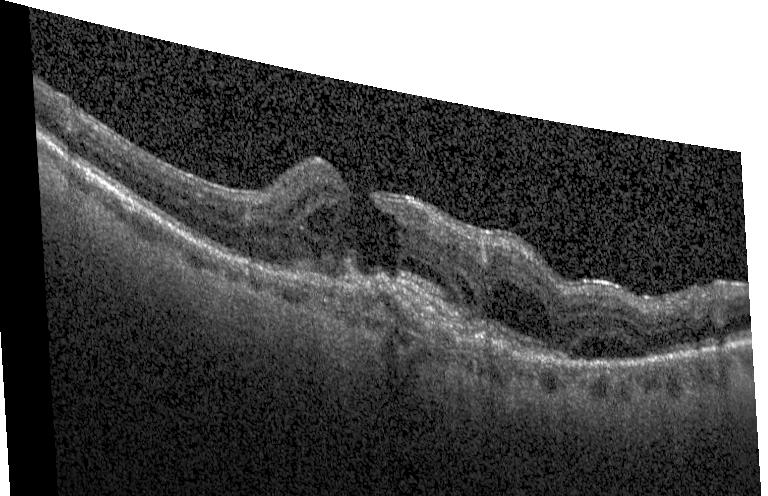
Assessment: a choroidal neovascular membrane.